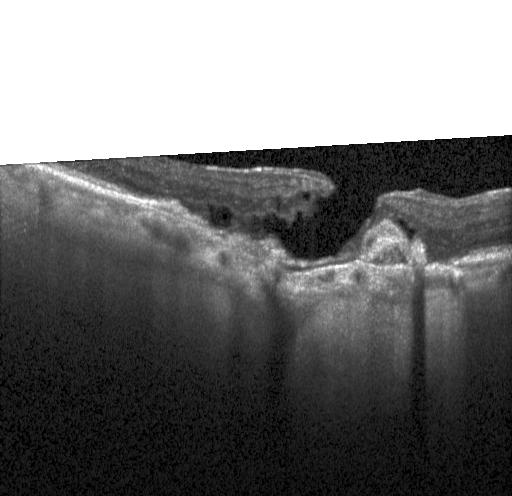 Heidelberg Spectralis · optical coherence tomography B-scan. Impression: CNV.